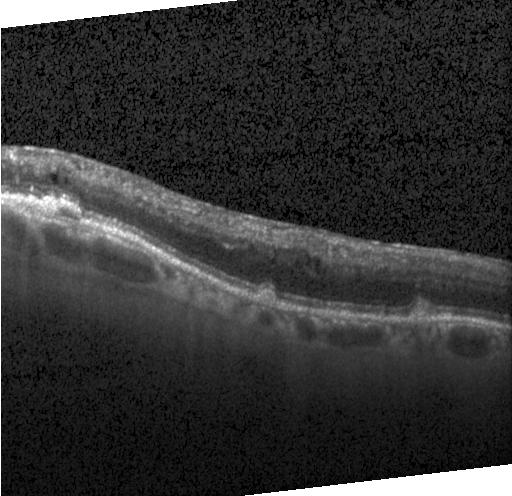

Centered on the fovea · OCT B-scan · acquired on a Heidelberg Spectralis
Finding: a choroidal neovascular membrane.